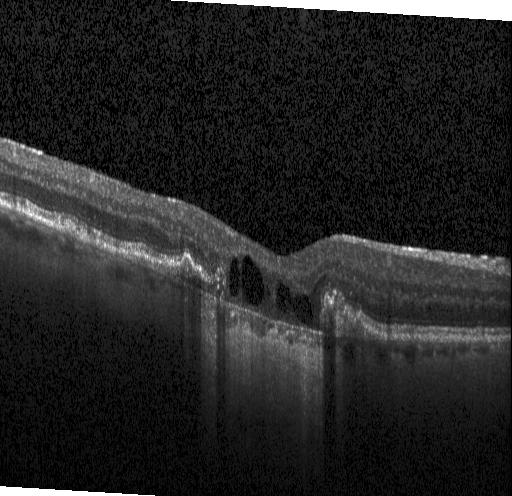
Retinal OCT cross-section; horizontal scan through the fovea
Dx: a choroidal neovascular membrane.